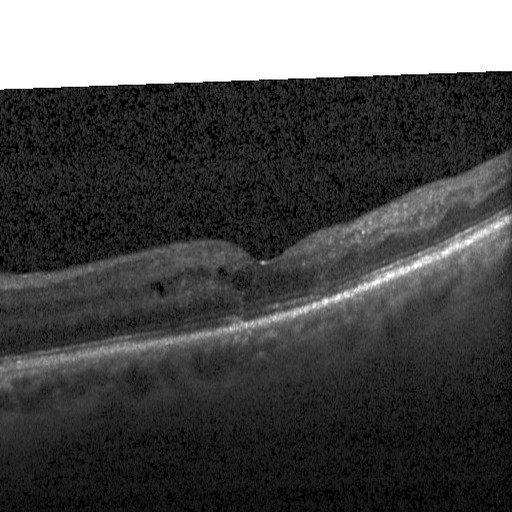
Dx: diabetic macular edema.